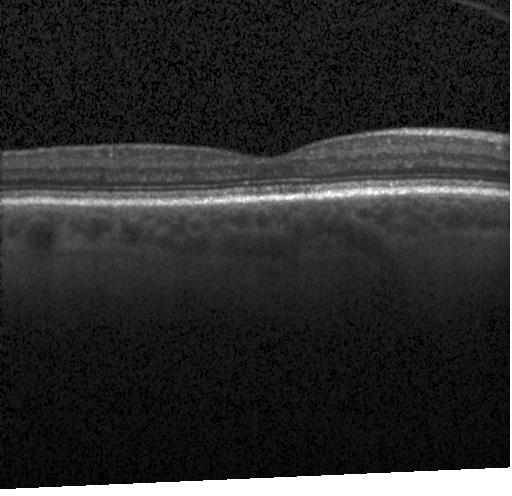
This B-scan demonstrates no CNV, DME, or drusen.